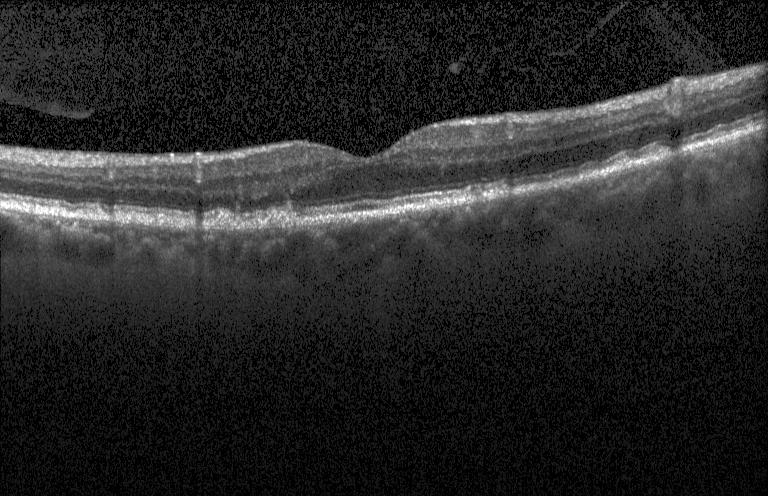 Dx: drusen.